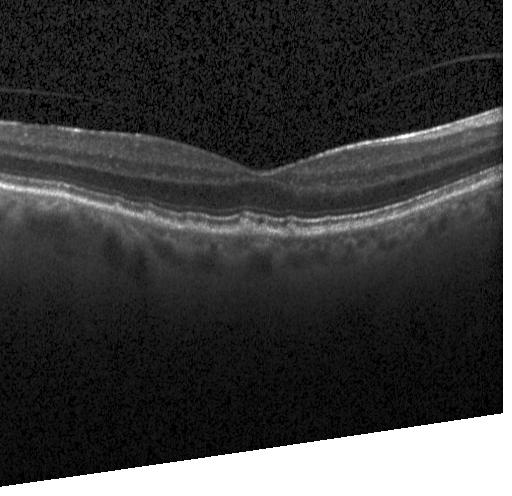
Impression: sub-RPE drusenoid deposits.